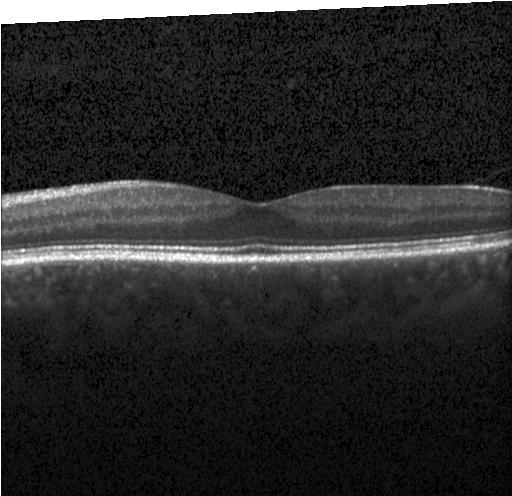 Macular OCT: neither choroidal neovascularization, diabetic macular edema, nor drusen.